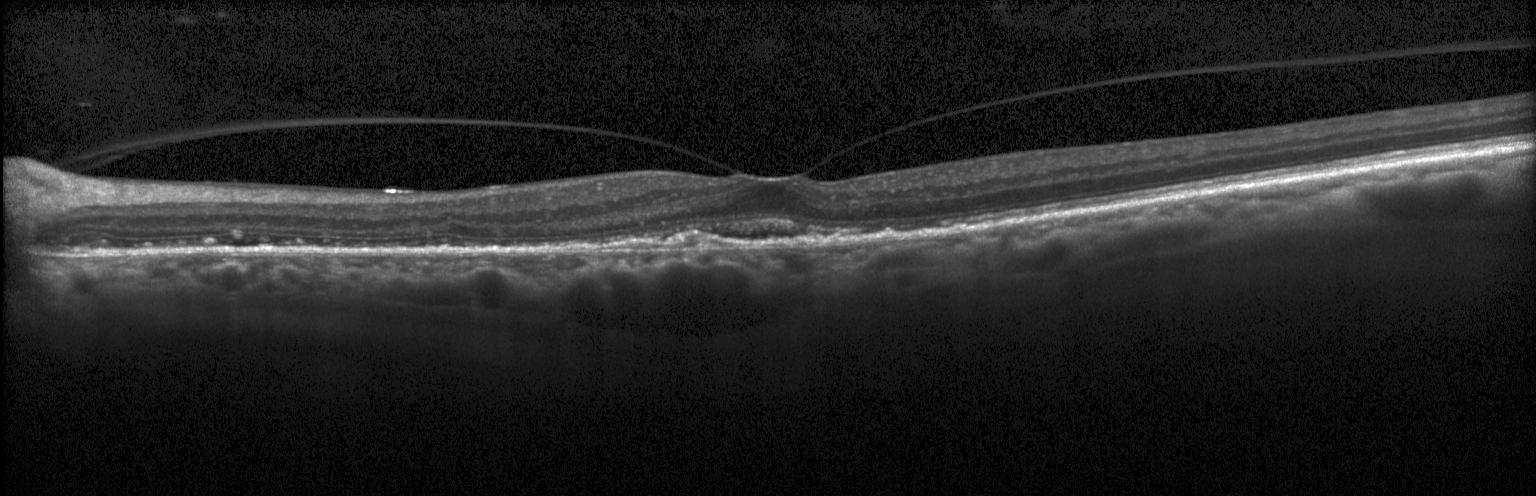

Finding: choroidal neovascularization (CNV).